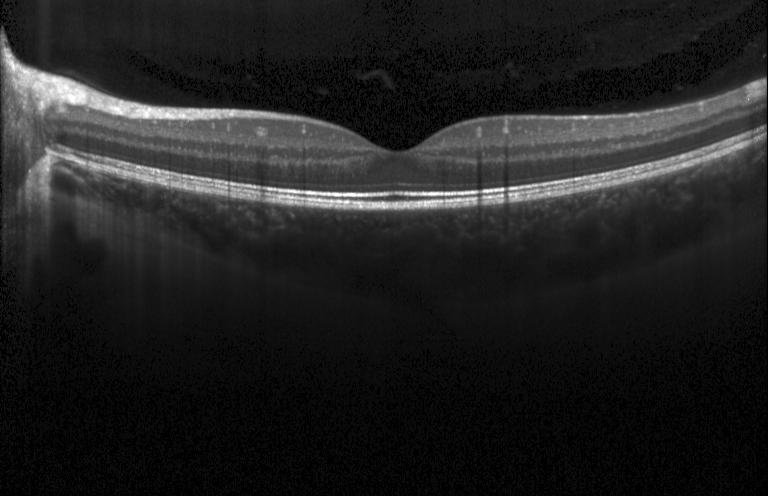 OCT line scan. Through the macula. Spectral-domain optical coherence tomography. Heidelberg Spectralis OCT system — No choroidal neovascularization, no diabetic macular edema, and no drusen.